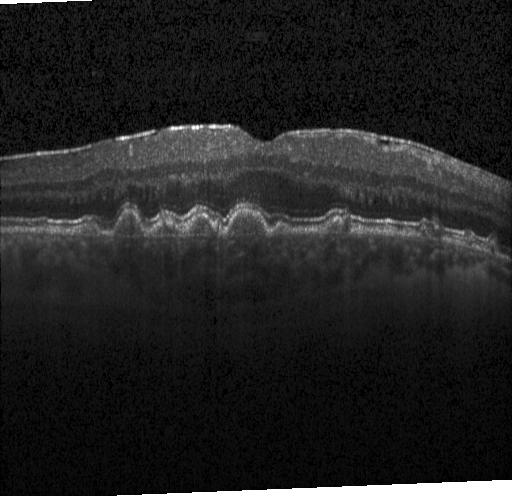
Optical coherence tomography B-scan · spectral-domain optical coherence tomography · acquired on a Heidelberg Spectralis · fovea-centered.
OCT finding: drusen.